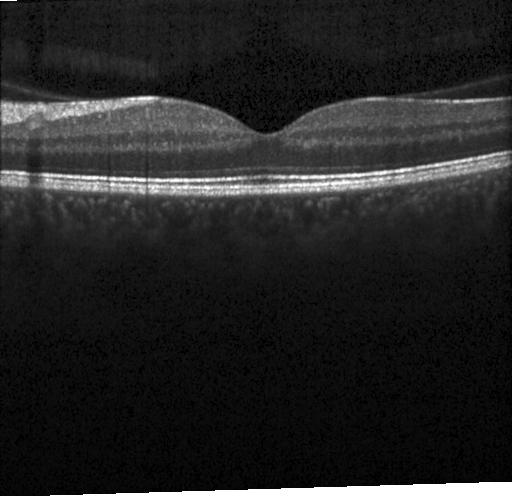 OCT scan showing no evidence of choroidal neovascularization, diabetic macular edema, or drusen.